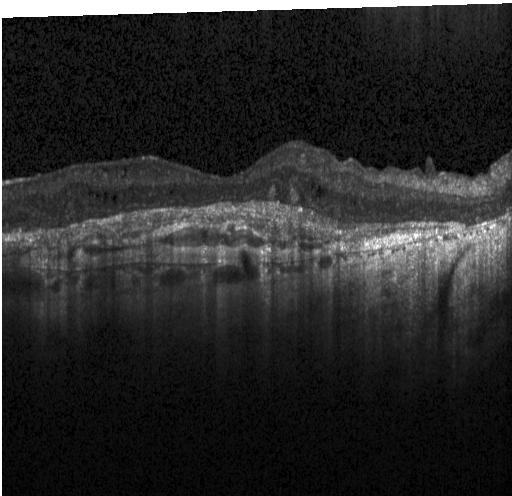

OCT B-scan showing CNV.